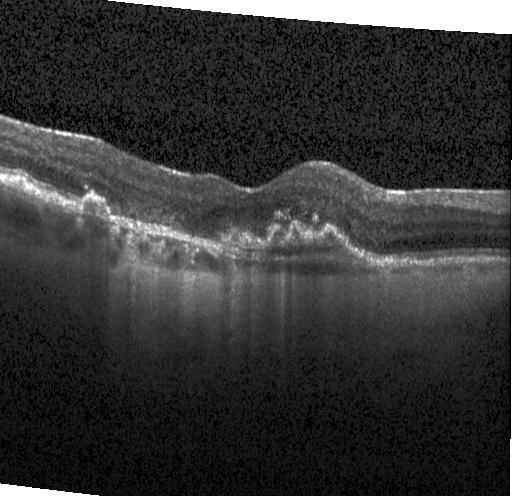
Retinal OCT B-scan. Spectral-domain optical coherence tomography. Horizontal scan through the fovea. Heidelberg Spectralis OCT system.
This B-scan demonstrates a choroidal neovascular membrane.